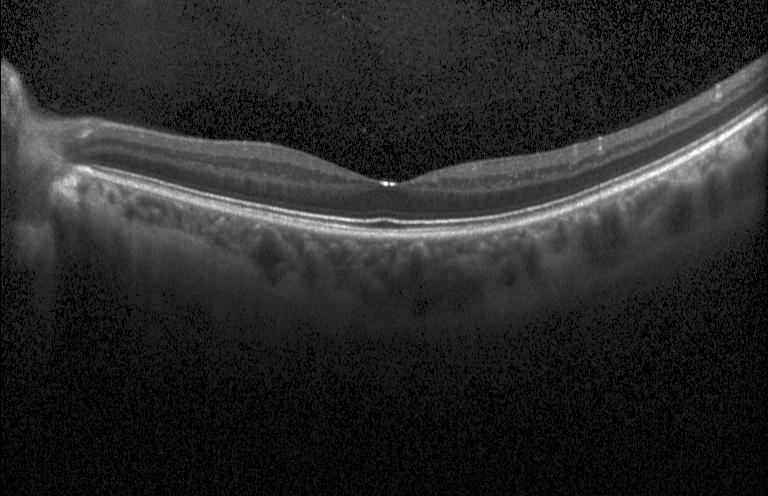 Heidelberg Spectralis OCT system; OCT line scan — Assessment: no choroidal neovascularization, diabetic macular edema, or drusen.